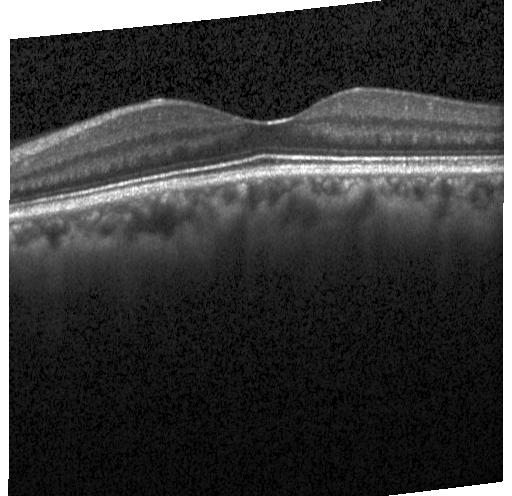

Spectral-domain optical coherence tomography · acquired on a Heidelberg Spectralis · fovea-centered · optical coherence tomography scan.
The scan shows no choroidal neovascularization, diabetic macular edema, or drusen.